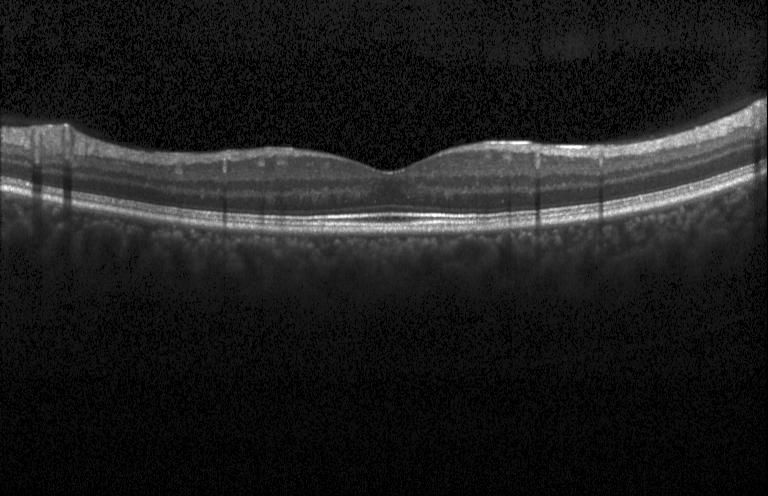 No evidence of choroidal neovascularization, diabetic macular edema, or drusen.